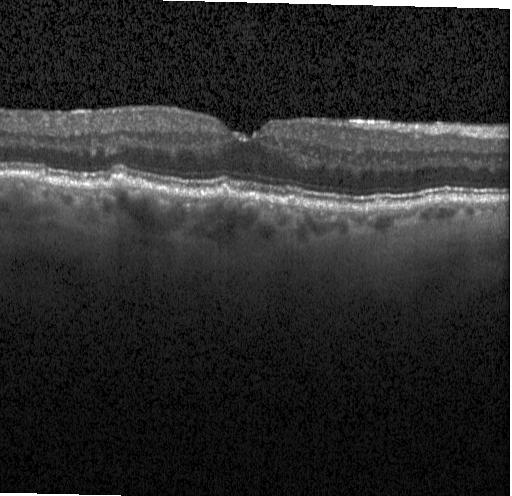 Macular OCT: multiple drusen.